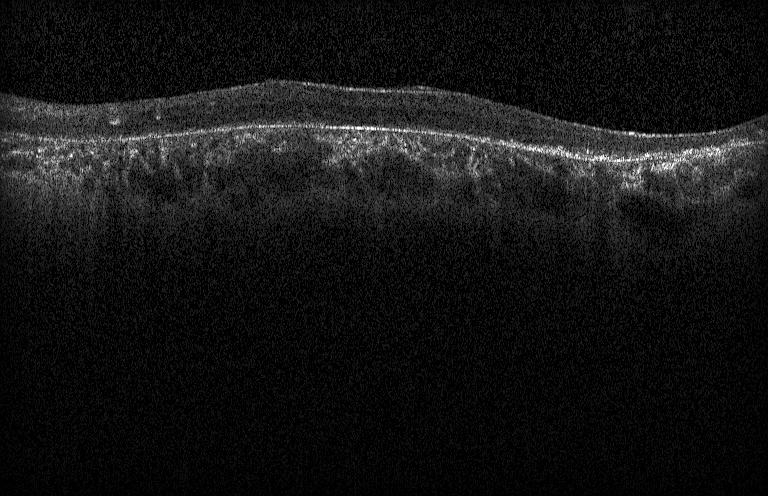 OCT B-scan. SD-OCT.
Diagnosis: no CNV, no DME, and no drusen.